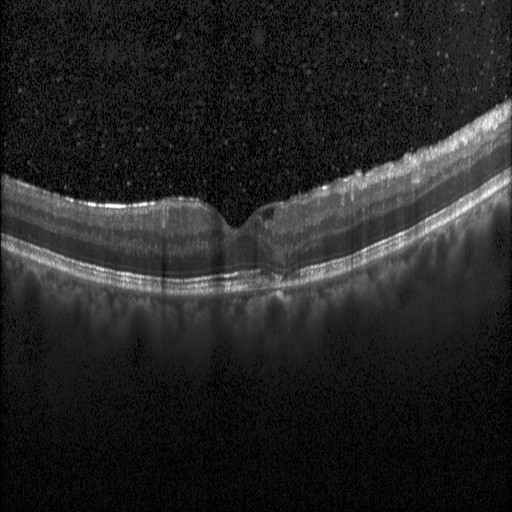 Centered on the fovea; instrument: Heidelberg Spectralis; optical coherence tomography B-scan — Diagnosis: DME.